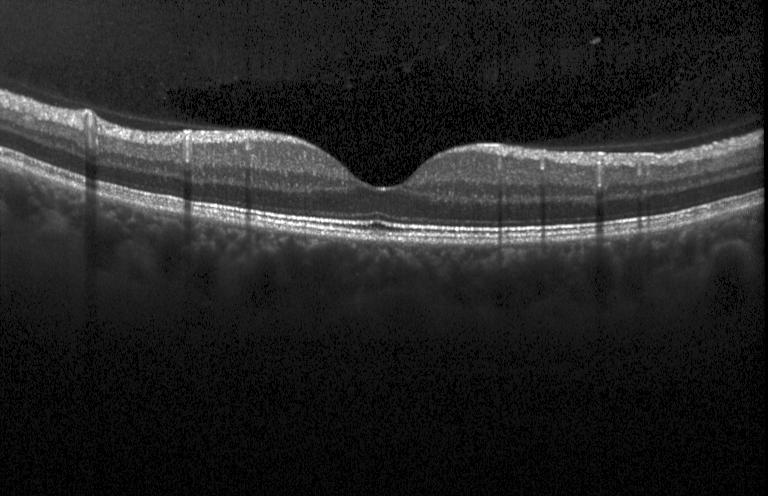 Optical coherence tomography B-scan — Finding: neither CNV, DME, nor drusen.